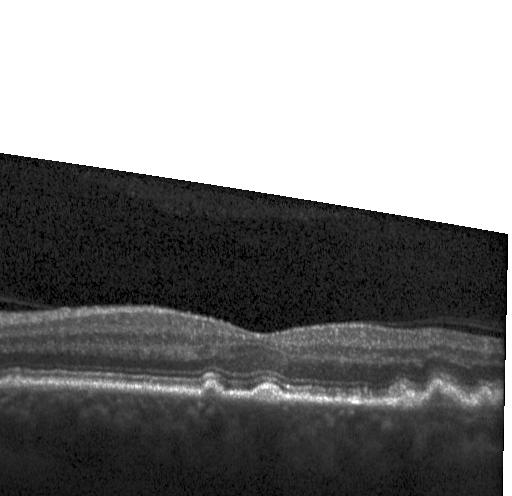
Spectral-domain optical coherence tomography · instrument: Heidelberg Spectralis · OCT B-scan · centered on the fovea
Impression: sub-RPE drusenoid deposits.